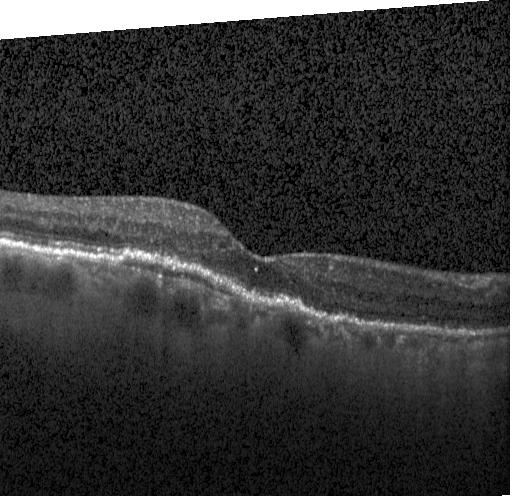
Retinal OCT cross-section. Heidelberg Spectralis OCT system — Assessment: CNV.